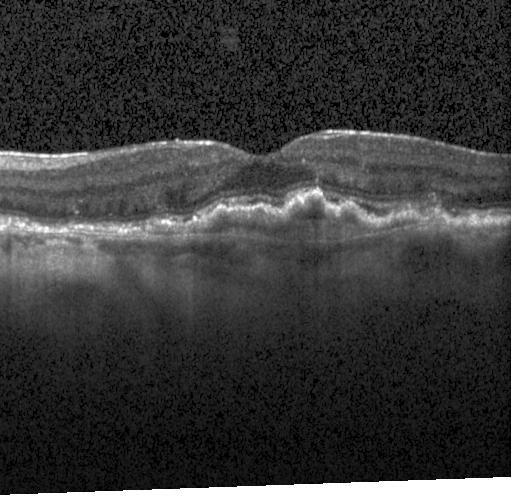 Spectral-domain OCT · retinal OCT cross-section. Macular OCT: a choroidal neovascular membrane.